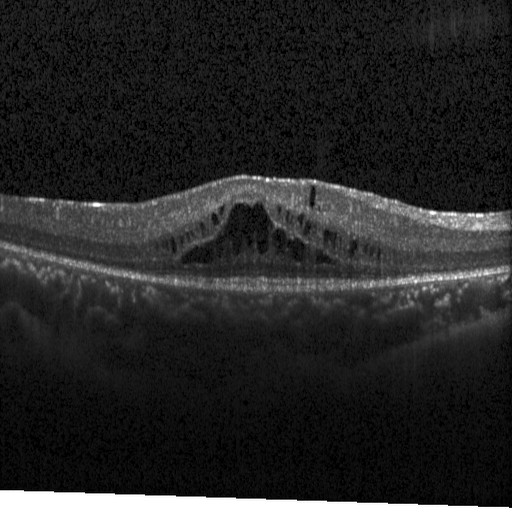 Macular scan; optical coherence tomography B-scan; acquired on a Heidelberg Spectralis.
Impression: diabetic macular edema.